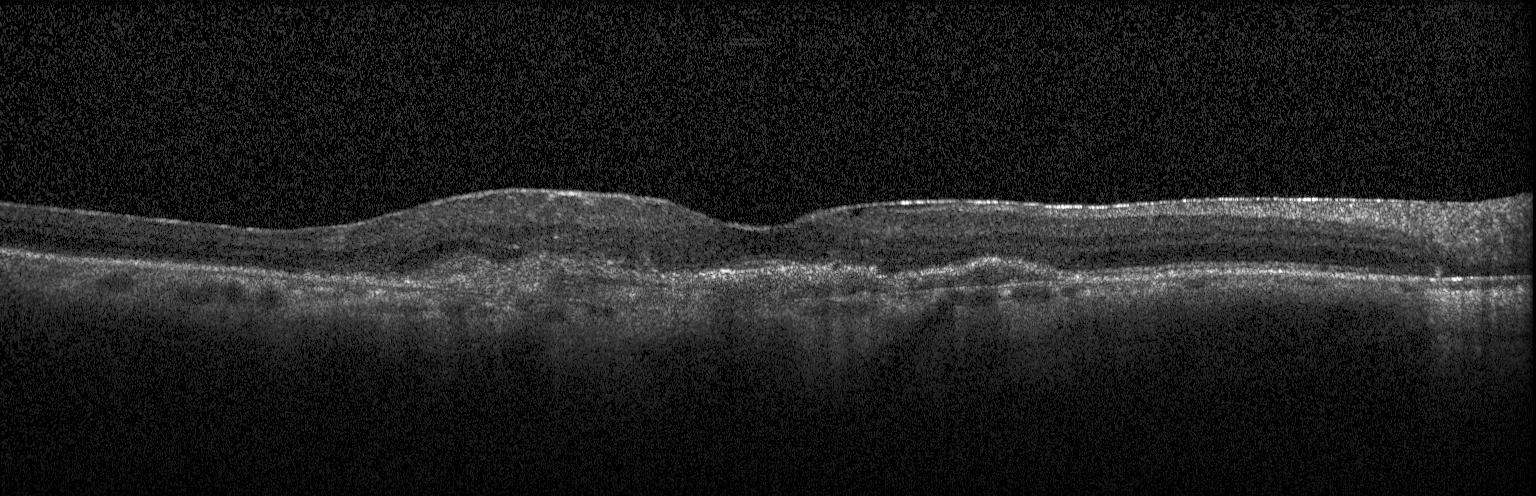 Instrument: Heidelberg Spectralis, OCT line scan, SD-OCT, macular scan
This B-scan demonstrates CNV.